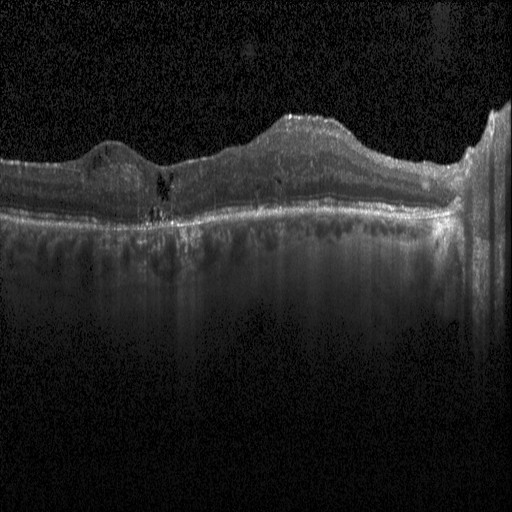

Horizontal scan through the fovea, SD-OCT, retinal OCT B-scan.
Finding: diabetic macular edema.